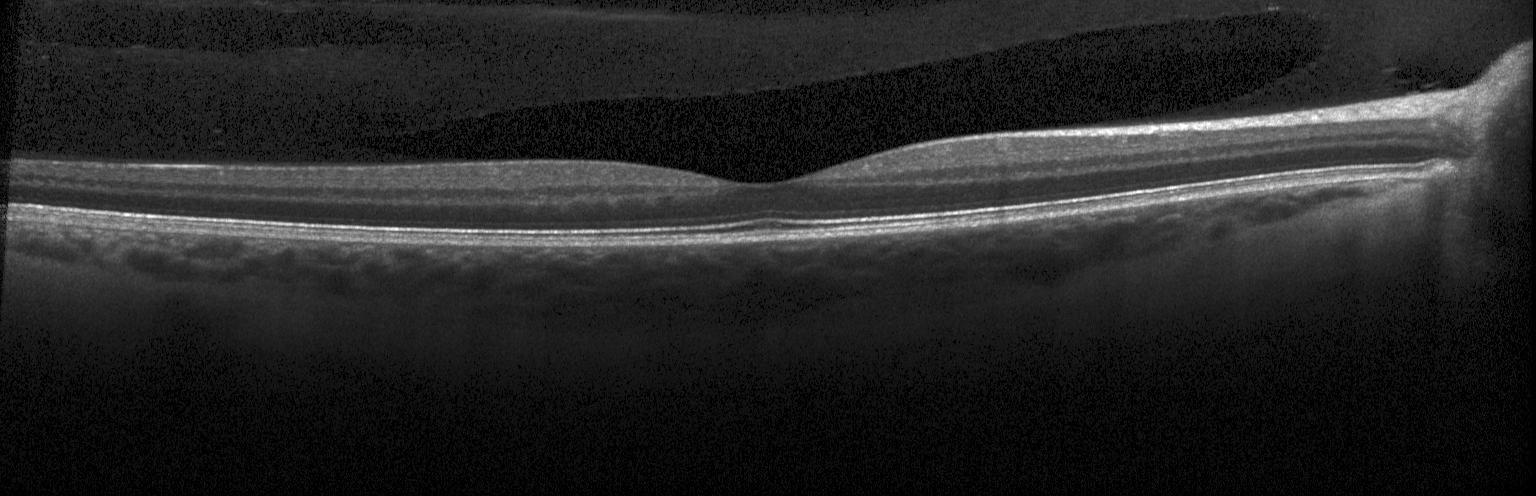
Assessment: no choroidal neovascularization, diabetic macular edema, or drusen.